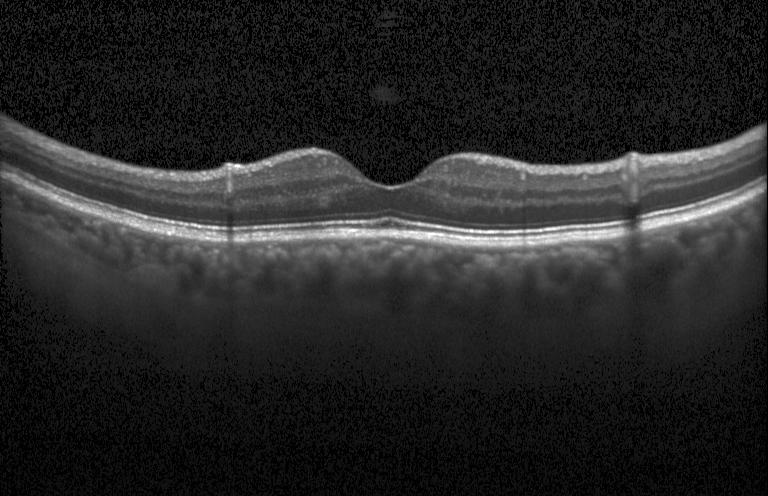
Spectral-domain OCT B-scan: no choroidal neovascularization, diabetic macular edema, or drusen.